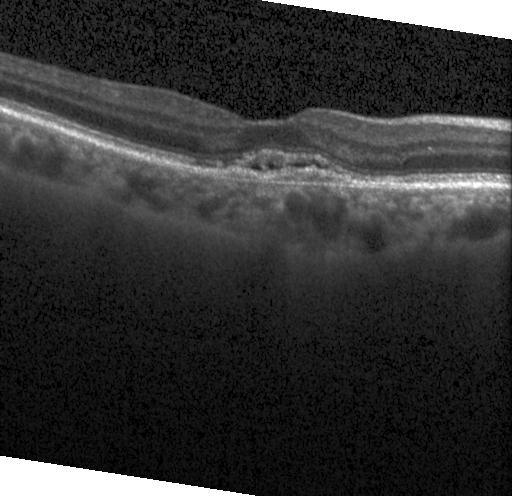
Centered on the fovea; OCT line scan.
A choroidal neovascular membrane.